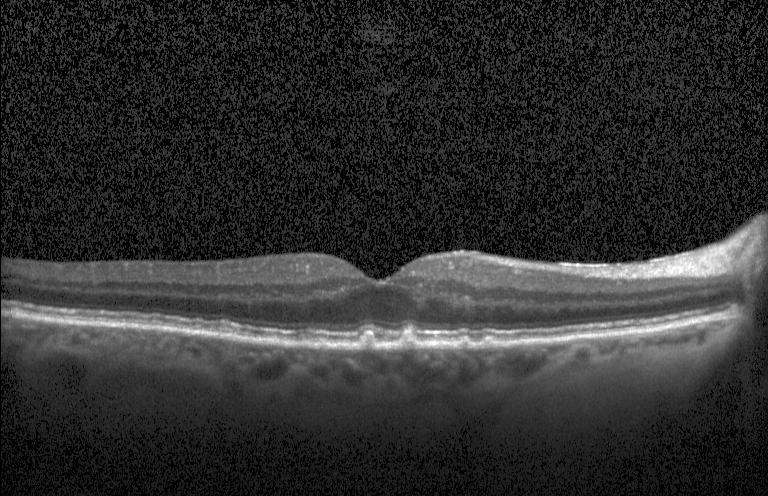
OCT line scan, SD-OCT — Sub-RPE drusenoid deposits.